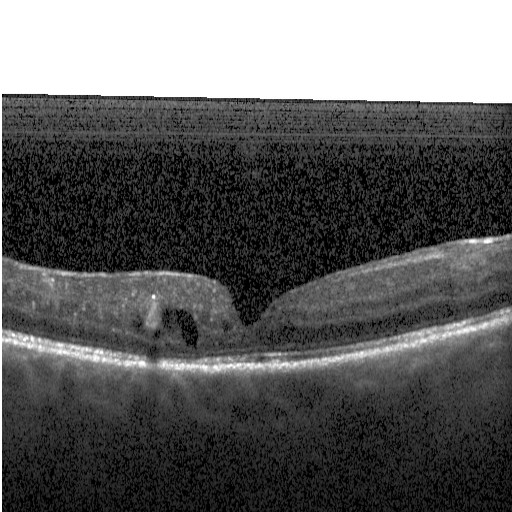 Heidelberg Spectralis OCT system; horizontal scan through the fovea; OCT B-scan; SD-OCT — Finding: DME.